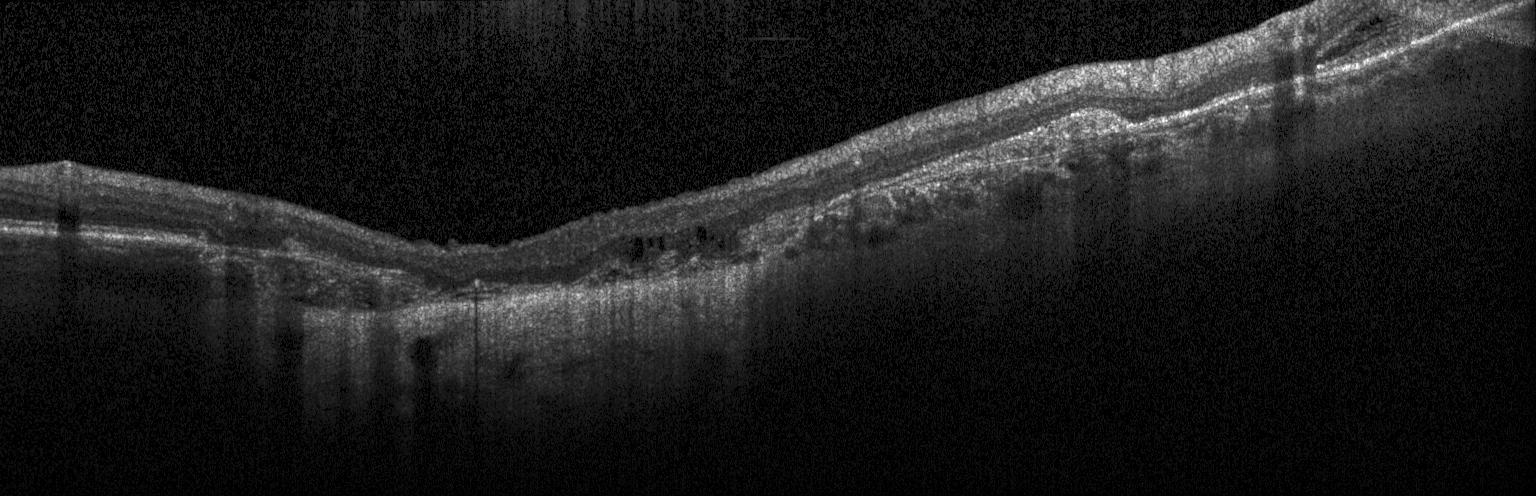 Optical coherence tomography scan.
Finding: a choroidal neovascular membrane.